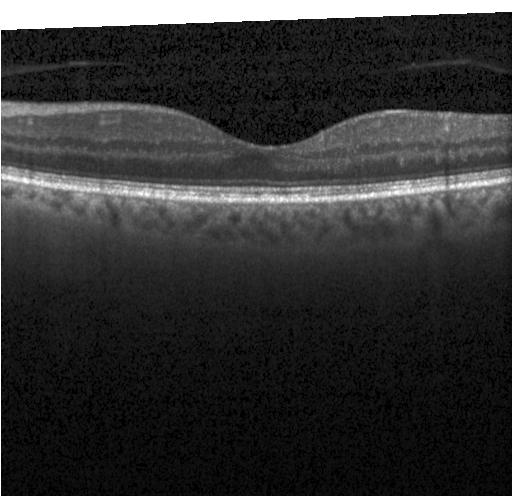 OCT scan showing neither choroidal neovascularization, diabetic macular edema, nor drusen.